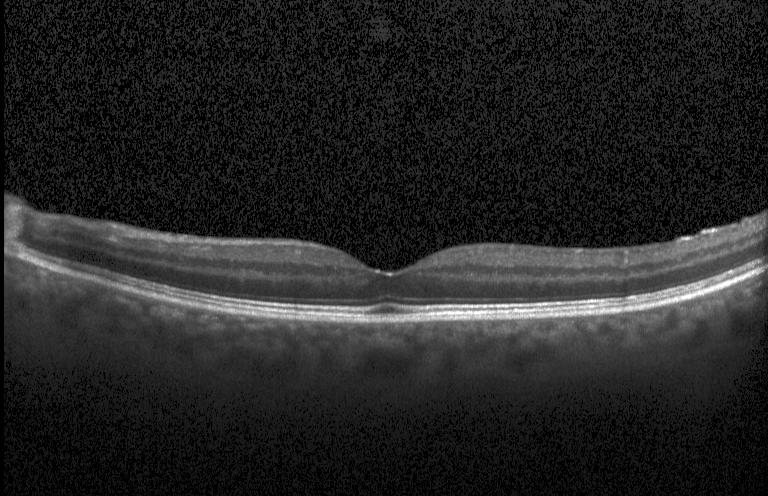
Retinal OCT cross-section, spectral-domain OCT, centered on the fovea, instrument: Heidelberg Spectralis — The scan shows no choroidal neovascularization, diabetic macular edema, or drusen.